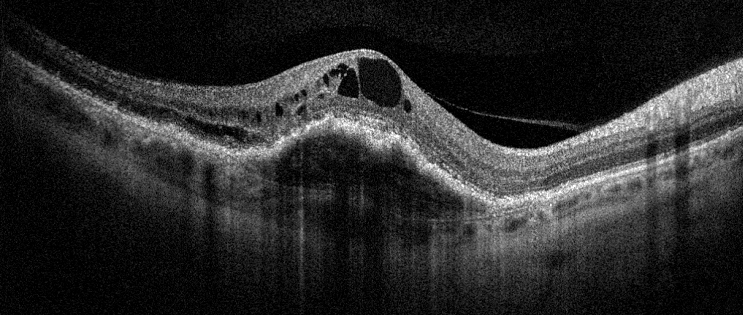 OCT B-scan; oculus dexter
Impression: AMD.